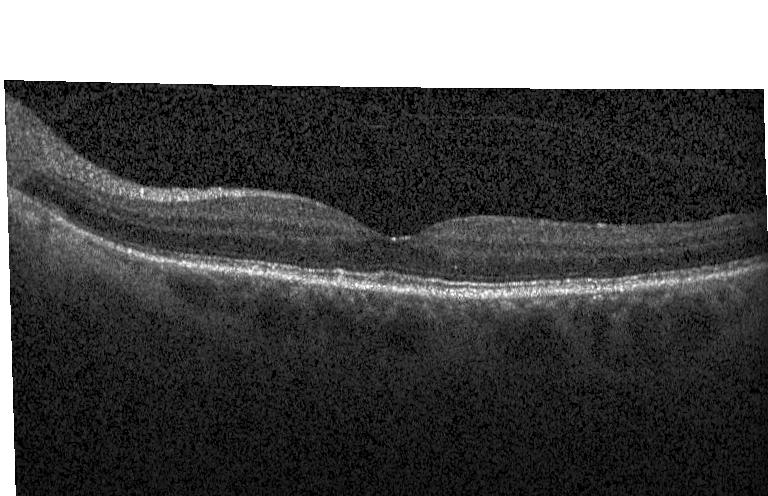
Retinal OCT cross-section.
Drusen.